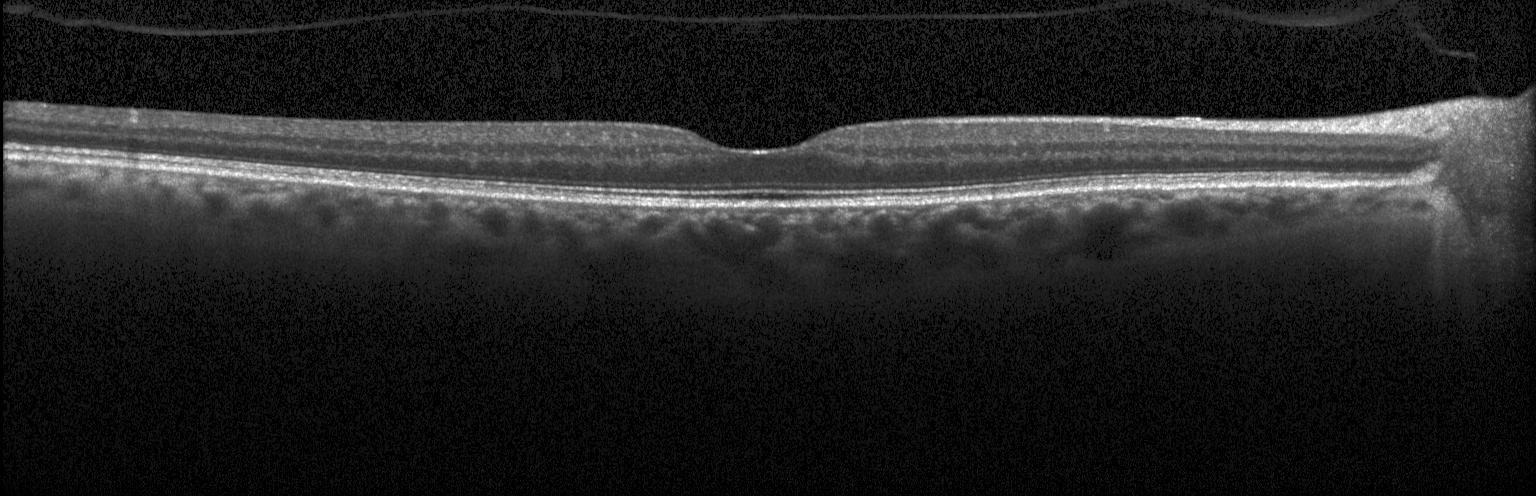 OCT line scan — Impression: no evidence of CNV, DME, or drusen.